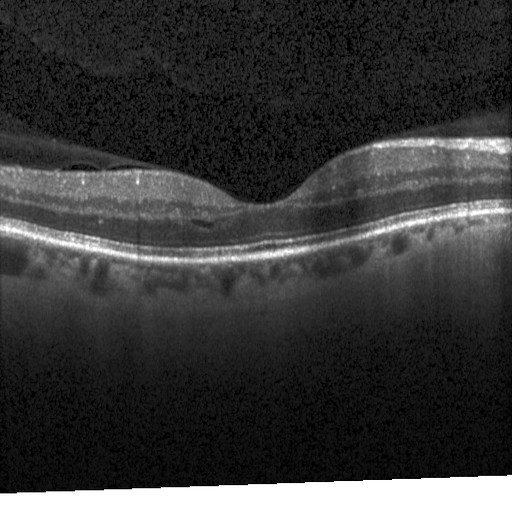
Optical coherence tomography scan; acquired on a Heidelberg Spectralis — Diagnosis: diabetic macular edema (DME).